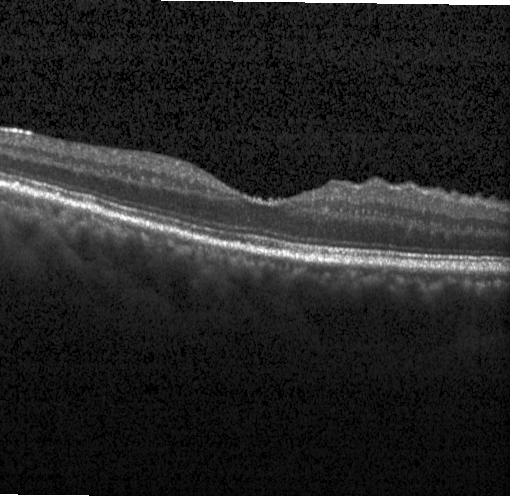

Retinal OCT cross-section. Centered on the fovea.
Neither CNV, DME, nor drusen.